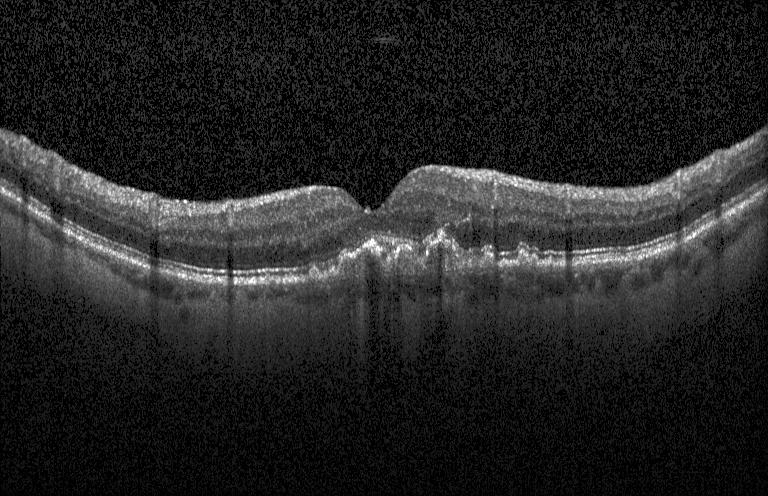
Impression: sub-RPE drusenoid deposits.